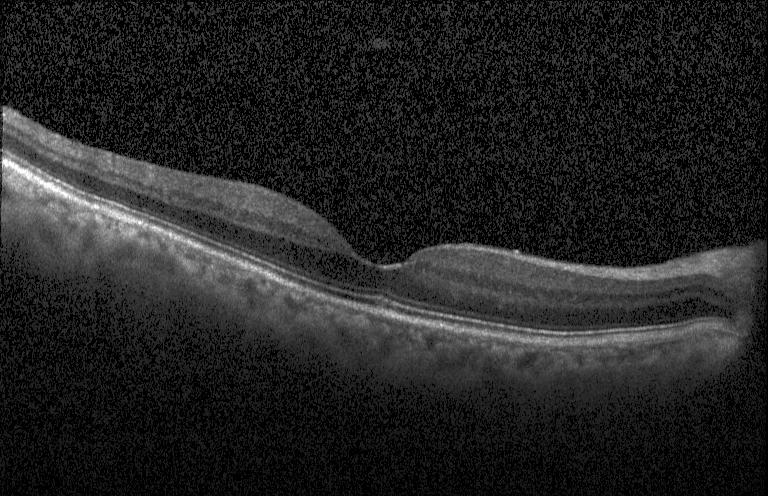 Spectral-domain optical coherence tomography · retinal OCT cross-section.
Finding: no choroidal neovascularization, diabetic macular edema, or drusen.